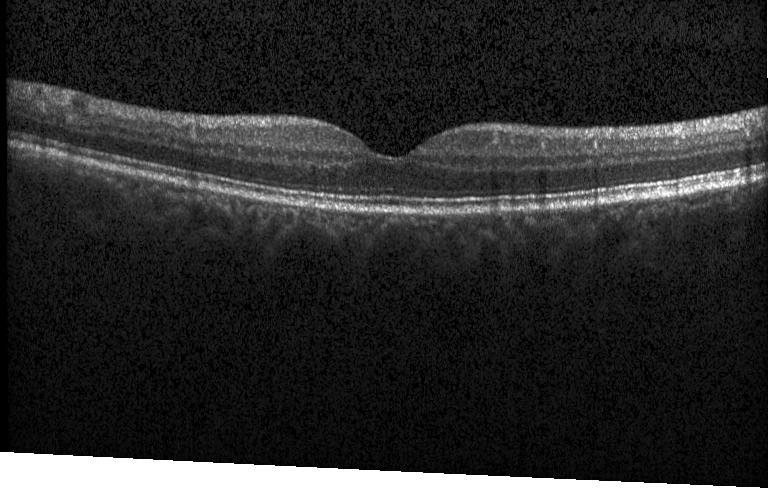 Retinal OCT cross-section.
OCT finding: no choroidal neovascularization, diabetic macular edema, or drusen.